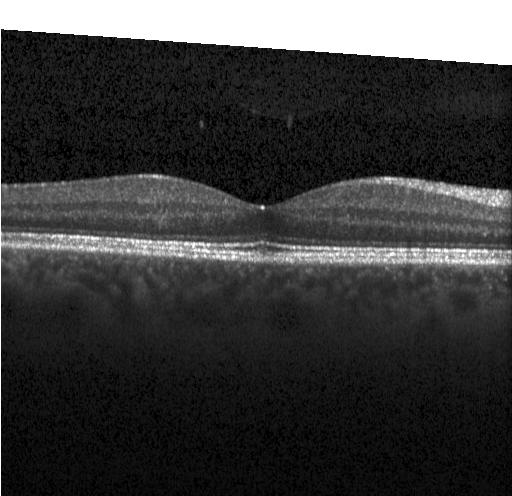

Retinal OCT cross-section showing no evidence of choroidal neovascularization, diabetic macular edema, or drusen.